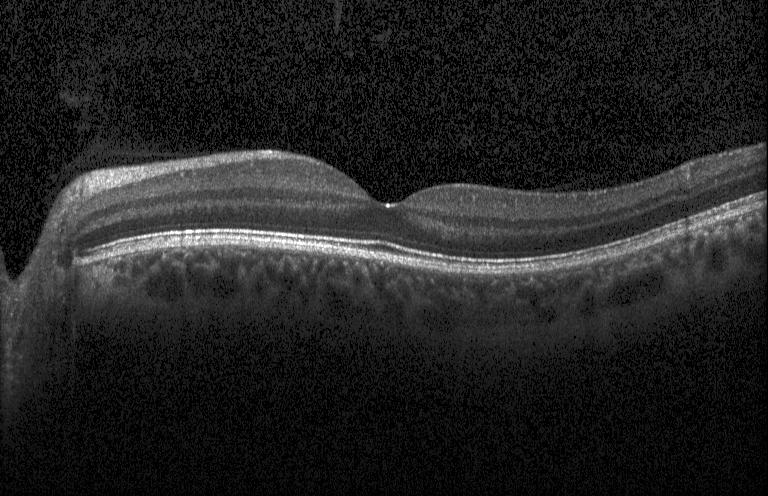
Spectral-domain OCT, acquired on a Heidelberg Spectralis, through the macula, OCT B-scan
Diagnosis: no choroidal neovascularization, no diabetic macular edema, and no drusen.